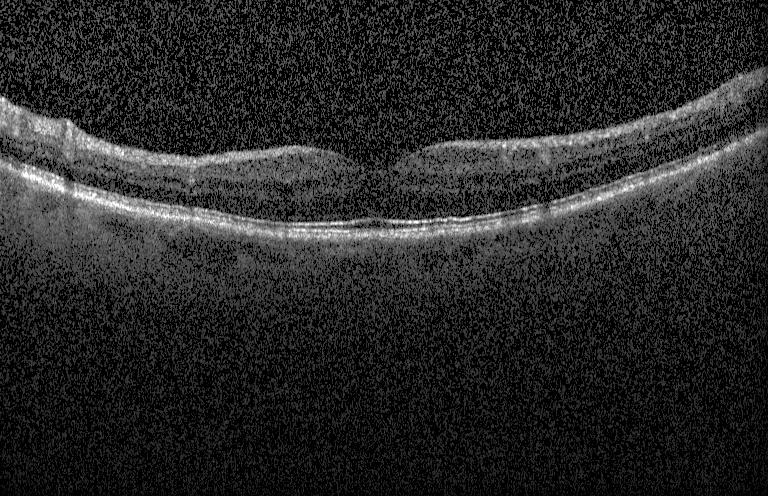

Finding: no choroidal neovascularization, no diabetic macular edema, and no drusen.